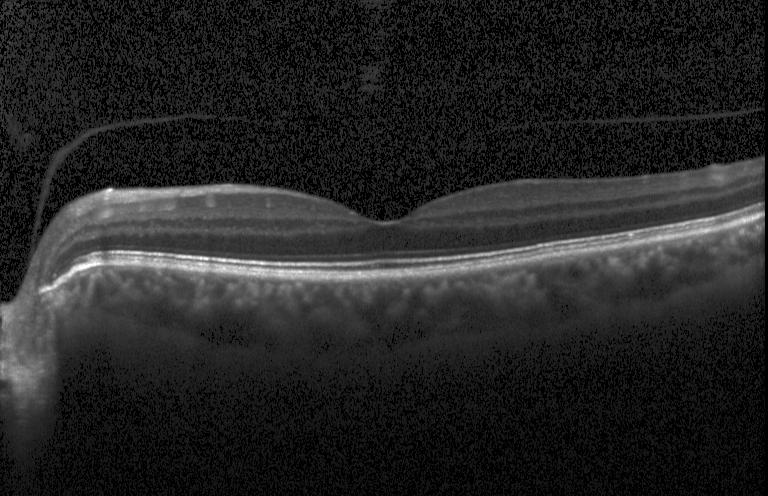

Optical coherence tomography scan, centered on the fovea
No choroidal neovascularization, diabetic macular edema, or drusen.